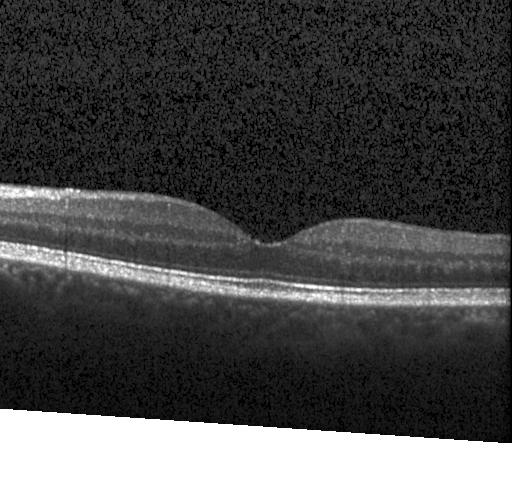 Finding: no evidence of CNV, DME, or drusen.